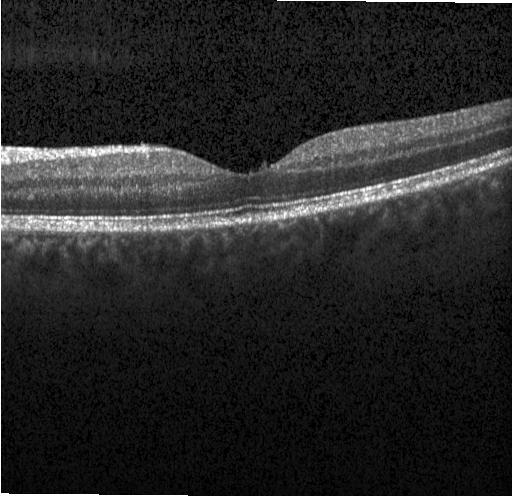
Diagnosis: no choroidal neovascularization, no diabetic macular edema, and no drusen.